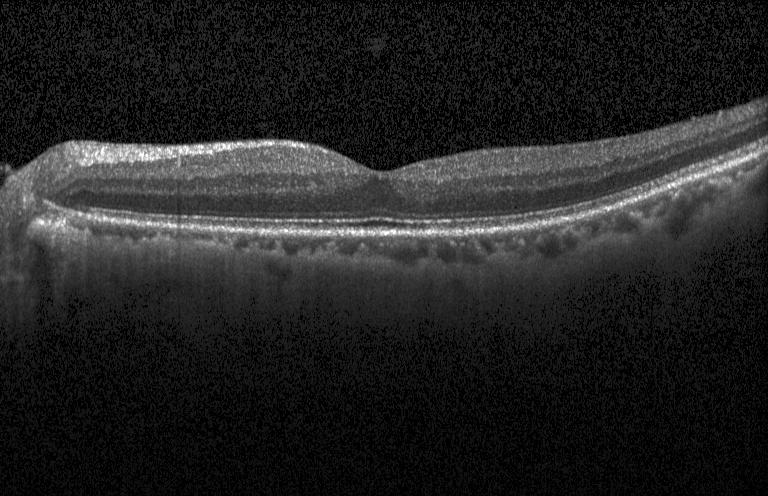

Retinal OCT cross-section showing no evidence of choroidal neovascularization, diabetic macular edema, or drusen.